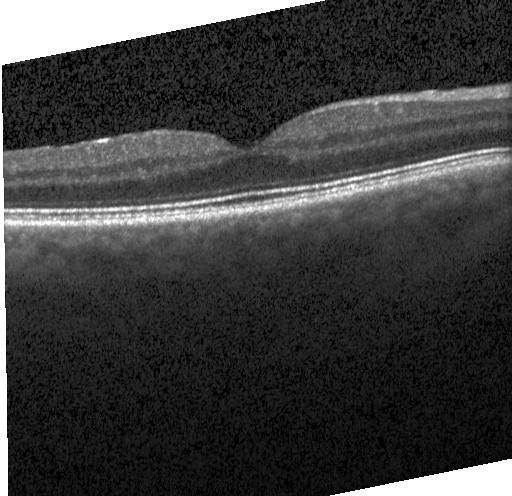

Macular OCT: neither choroidal neovascularization, diabetic macular edema, nor drusen.